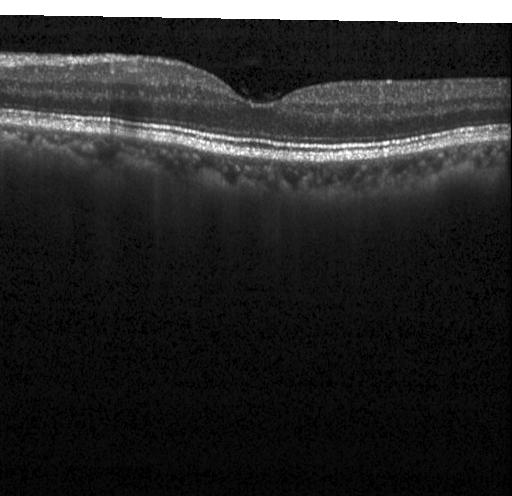
Retinal OCT cross-section · instrument: Heidelberg Spectralis · centered on the fovea · SD-OCT — Dx: neither choroidal neovascularization, diabetic macular edema, nor drusen.